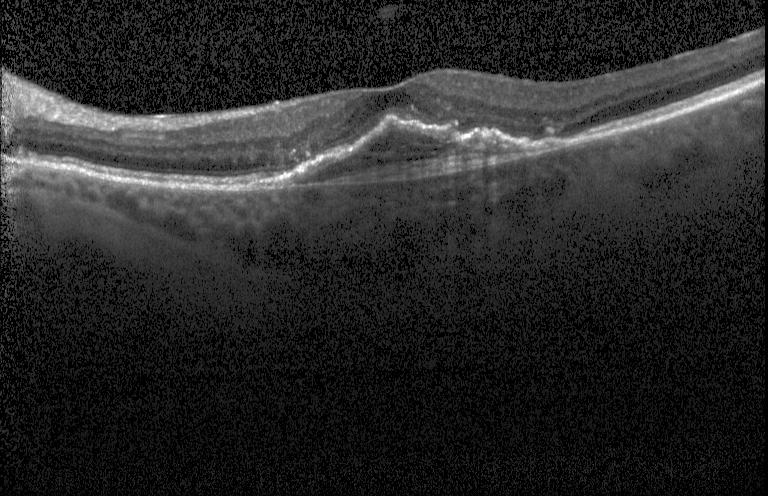 OCT B-scan, horizontal scan through the fovea.
This B-scan demonstrates choroidal neovascularization (CNV).